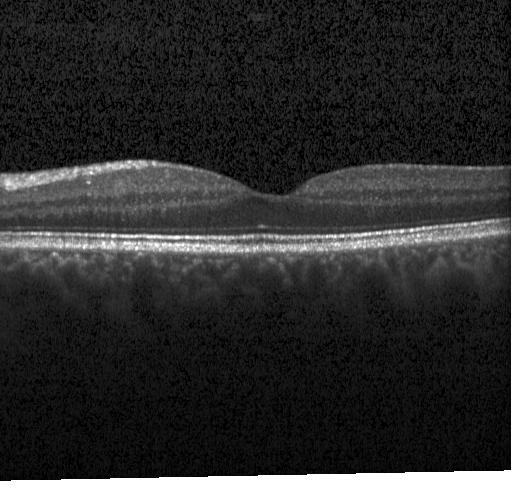

OCT line scan. Spectral-domain OCT. Instrument: Heidelberg Spectralis. Horizontal scan through the fovea
Assessment: no evidence of choroidal neovascularization, diabetic macular edema, or drusen.